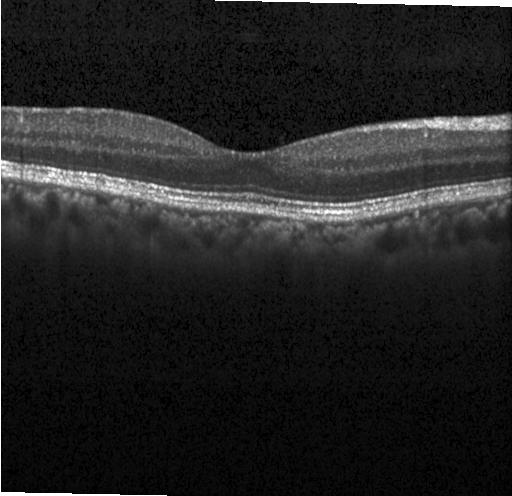
Acquired on a Heidelberg Spectralis; centered on the fovea; spectral-domain optical coherence tomography; retinal OCT B-scan
Assessment: neither choroidal neovascularization, diabetic macular edema, nor drusen.